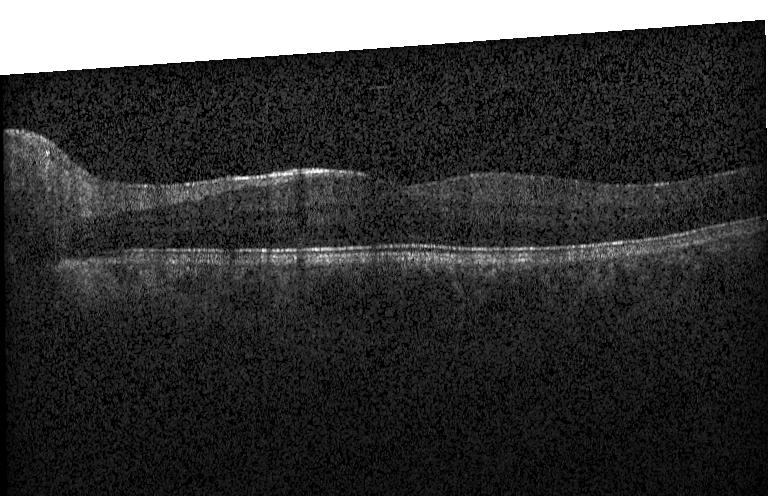

Optical coherence tomography scan; horizontal scan through the fovea; SD-OCT; Heidelberg Spectralis OCT system.
OCT finding: no choroidal neovascularization, no diabetic macular edema, and no drusen.